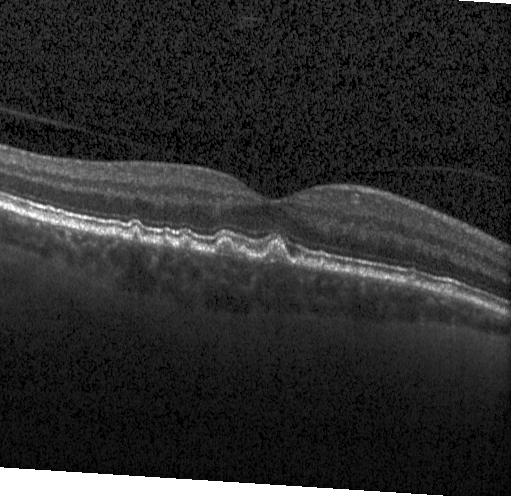
Spectral-domain OCT · instrument: Heidelberg Spectralis · optical coherence tomography B-scan · fovea-centered — Finding: multiple drusen.